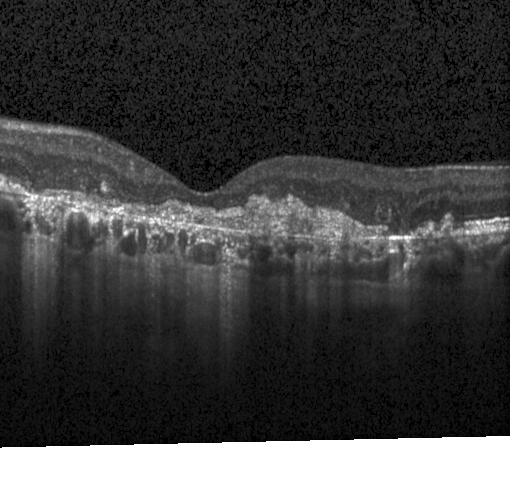 Through the macula; instrument: Heidelberg Spectralis; optical coherence tomography B-scan.
Impression: a choroidal neovascular membrane.